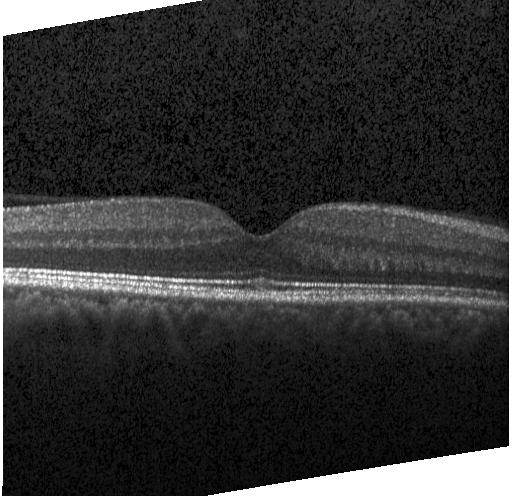

Finding: no evidence of choroidal neovascularization, diabetic macular edema, or drusen.